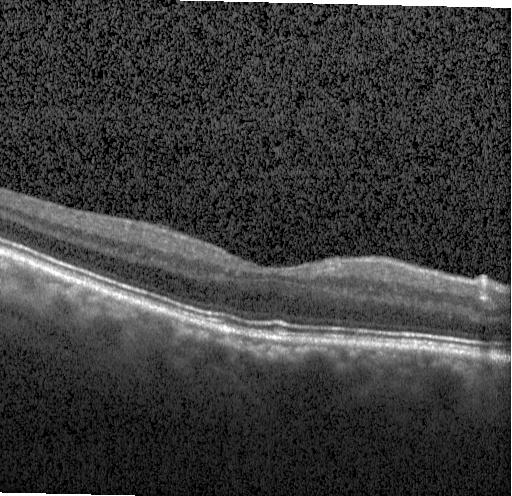
Centered on the fovea, instrument: Heidelberg Spectralis, spectral-domain optical coherence tomography, optical coherence tomography scan — Finding: sub-RPE drusenoid deposits.